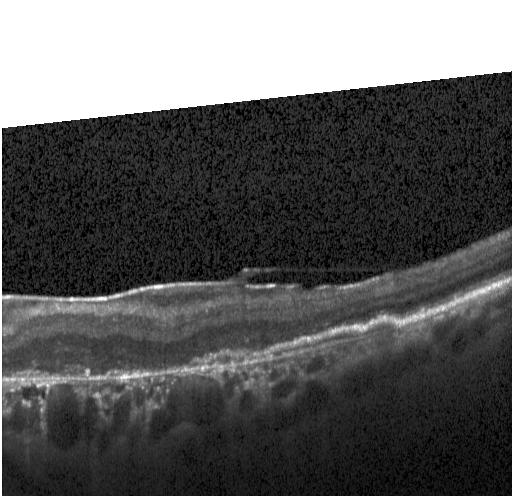 Instrument: Heidelberg Spectralis. Retinal OCT cross-section. Spectral-domain optical coherence tomography — Impression: CNV.